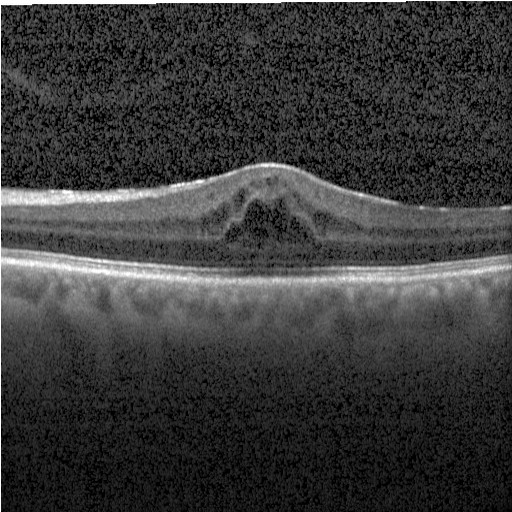
Centered on the fovea. Spectral-domain OCT. Retinal OCT B-scan.
Impression: diabetic macular edema.